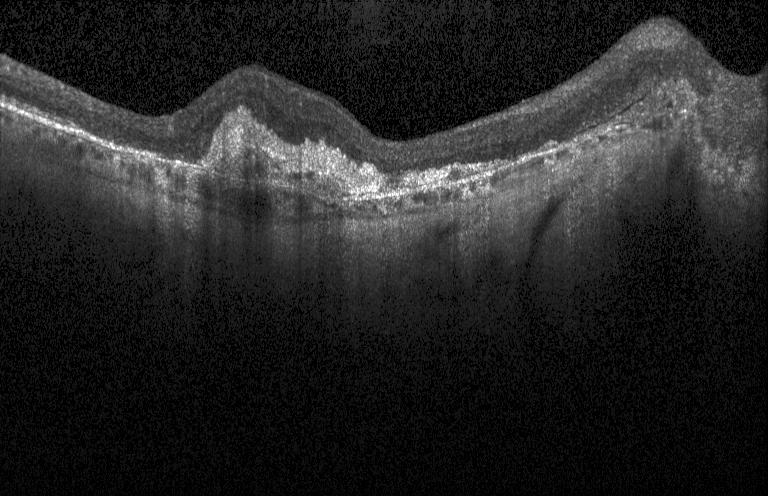
Retinal OCT B-scan, centered on the fovea.
Finding: choroidal neovascularization.